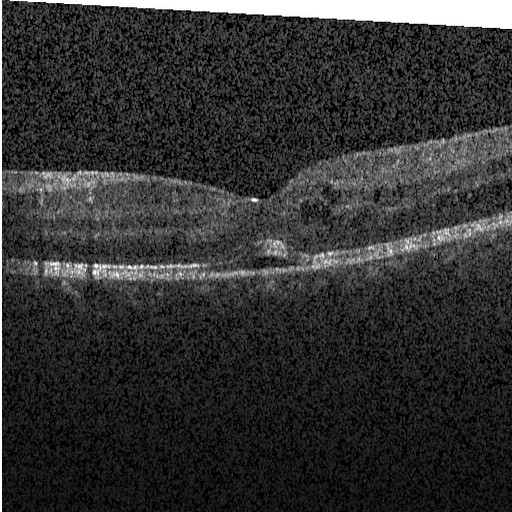 OCT scan showing diabetic macular edema (DME).